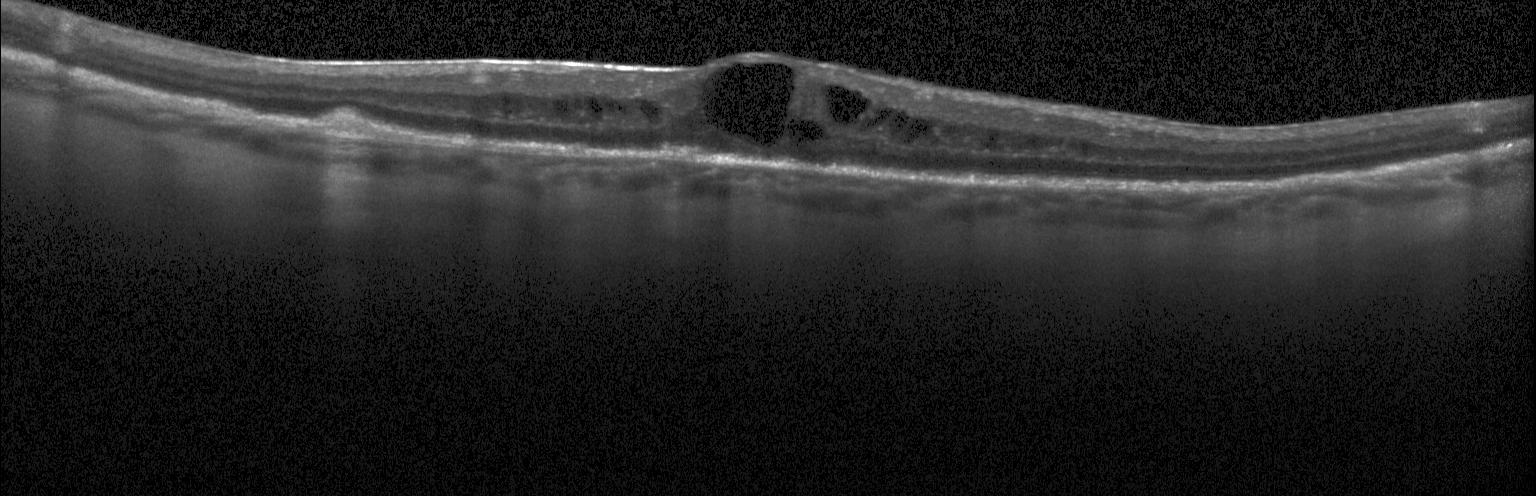 Retinal OCT cross-section
A choroidal neovascular membrane.